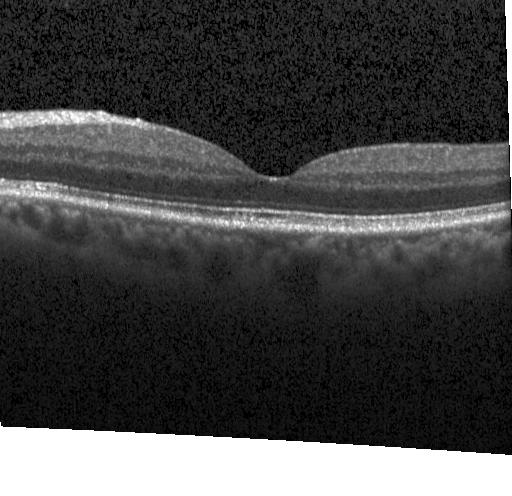
Impression: no evidence of choroidal neovascularization, diabetic macular edema, or drusen.